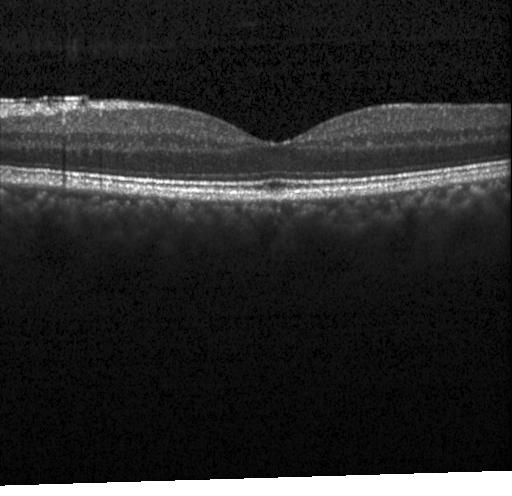

Optical coherence tomography scan.
Diagnosis: neither choroidal neovascularization, diabetic macular edema, nor drusen.